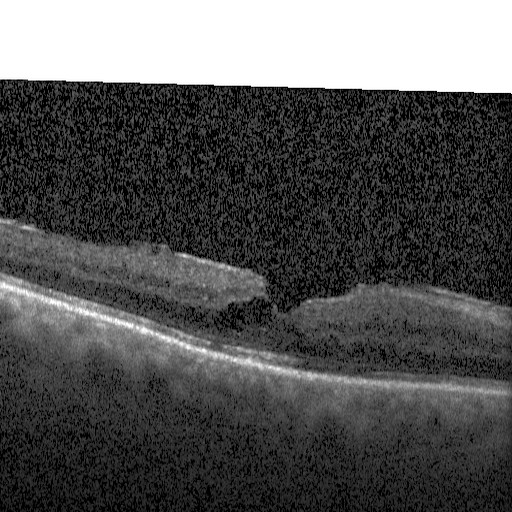
Spectral-domain optical coherence tomography. Optical coherence tomography scan.
Macular OCT: diabetic macular edema (DME).